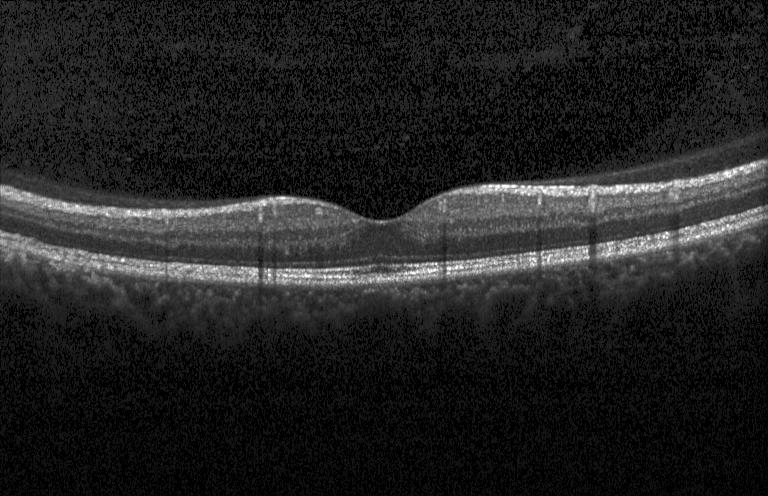 Through the macula, spectral-domain OCT, retinal OCT cross-section, acquired on a Heidelberg Spectralis.
Finding: no CNV, no DME, and no drusen.